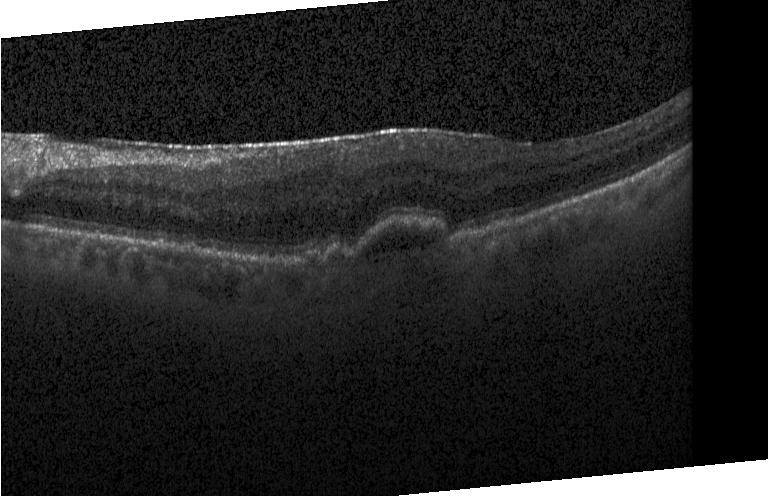

Optical coherence tomography B-scan, Heidelberg Spectralis OCT system, spectral-domain OCT — Diagnosis: a choroidal neovascular membrane.